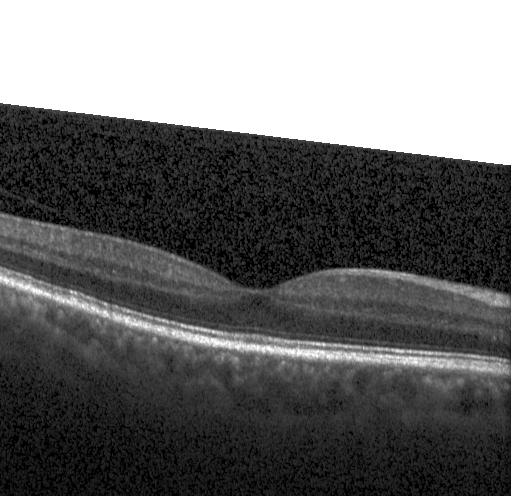 OCT B-scan. Heidelberg Spectralis. Spectral-domain OCT. Macular scan. This B-scan demonstrates no choroidal neovascularization, diabetic macular edema, or drusen.